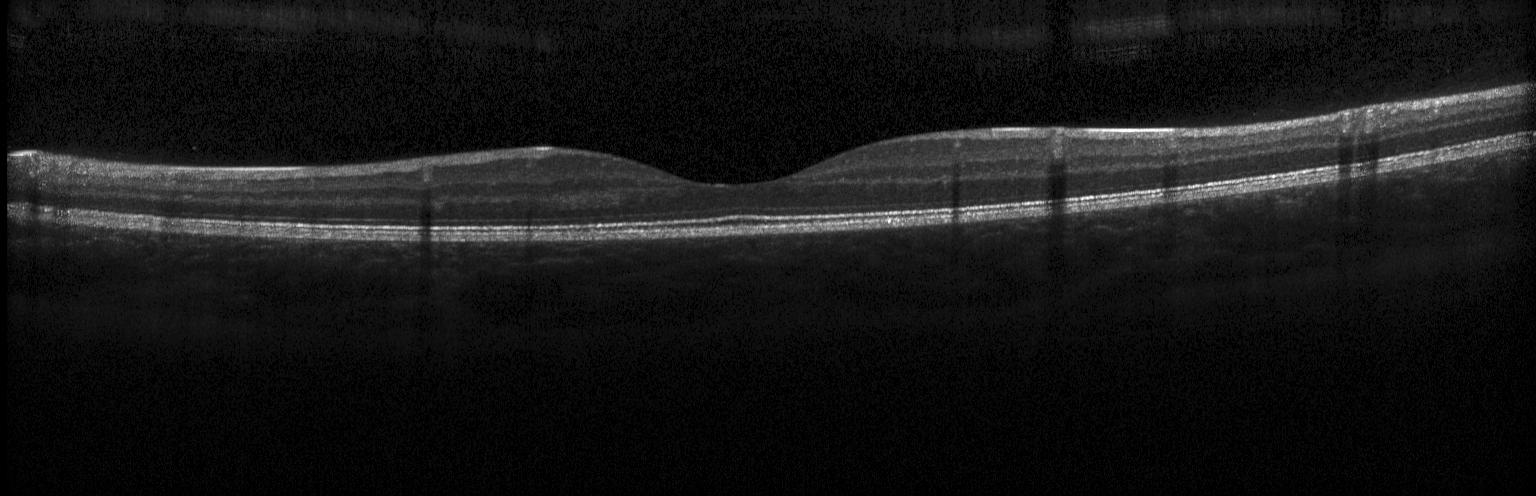

Optical coherence tomography scan. Diagnosis: no choroidal neovascularization, no diabetic macular edema, and no drusen.